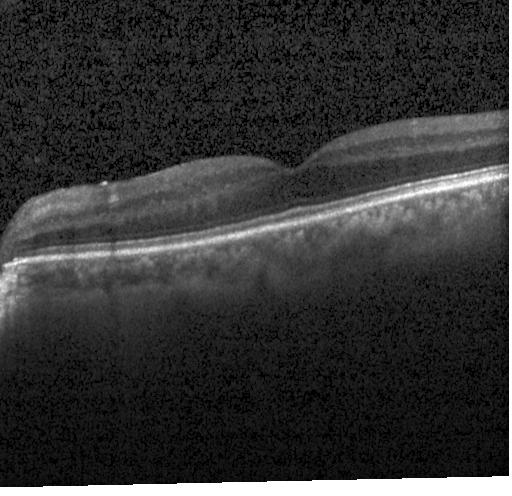 Optical coherence tomography B-scan; horizontal scan through the fovea; acquired on a Heidelberg Spectralis. Finding: neither choroidal neovascularization, diabetic macular edema, nor drusen.